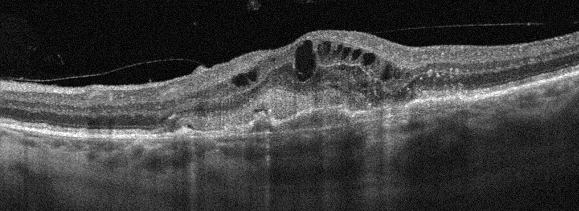 Oculus sinister, fovea-centered, Optovue Avanti RTVue XR, optical coherence tomography B-scan — The scan shows age-related macular degeneration.